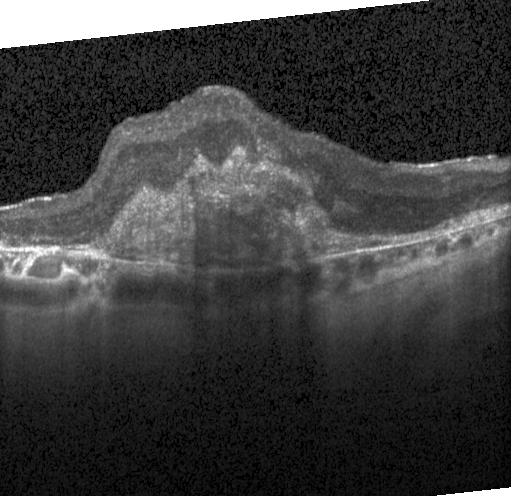 Finding: choroidal neovascularization (CNV).